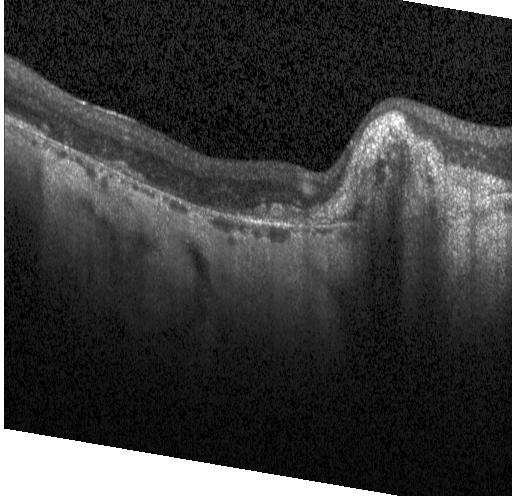

Retinal OCT cross-section, spectral-domain optical coherence tomography.
The scan shows choroidal neovascularization.